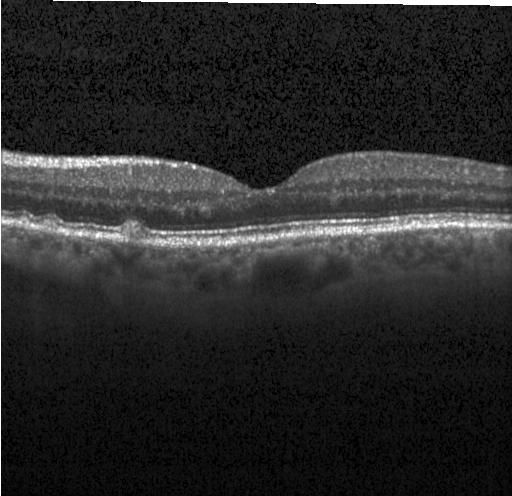
Sub-RPE drusenoid deposits.